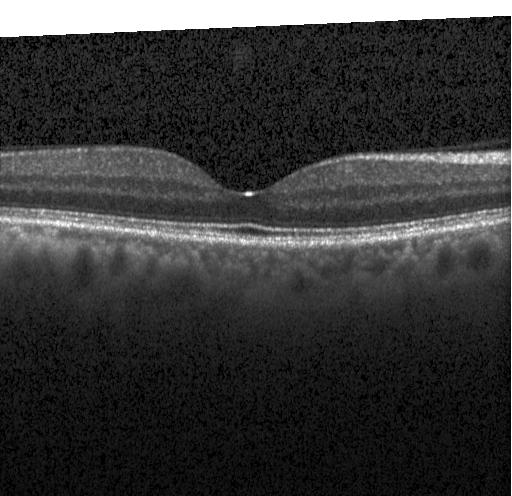

Spectral-domain optical coherence tomography · OCT B-scan · fovea-centered · instrument: Heidelberg Spectralis
No evidence of CNV, DME, or drusen.